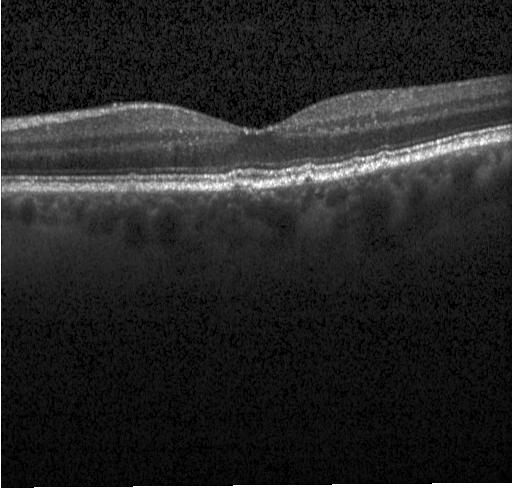

Finding: drusen.